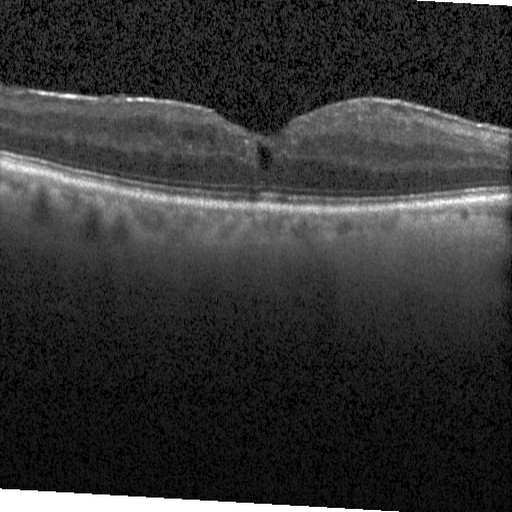
Spectral-domain OCT B-scan: DME.